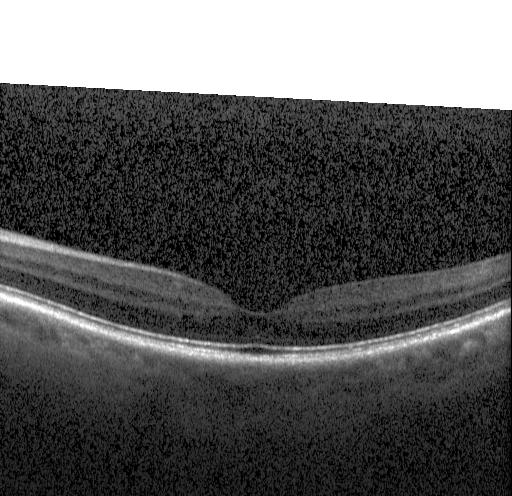

Spectral-domain OCT; Heidelberg Spectralis; OCT B-scan. Assessment: no evidence of choroidal neovascularization, diabetic macular edema, or drusen.